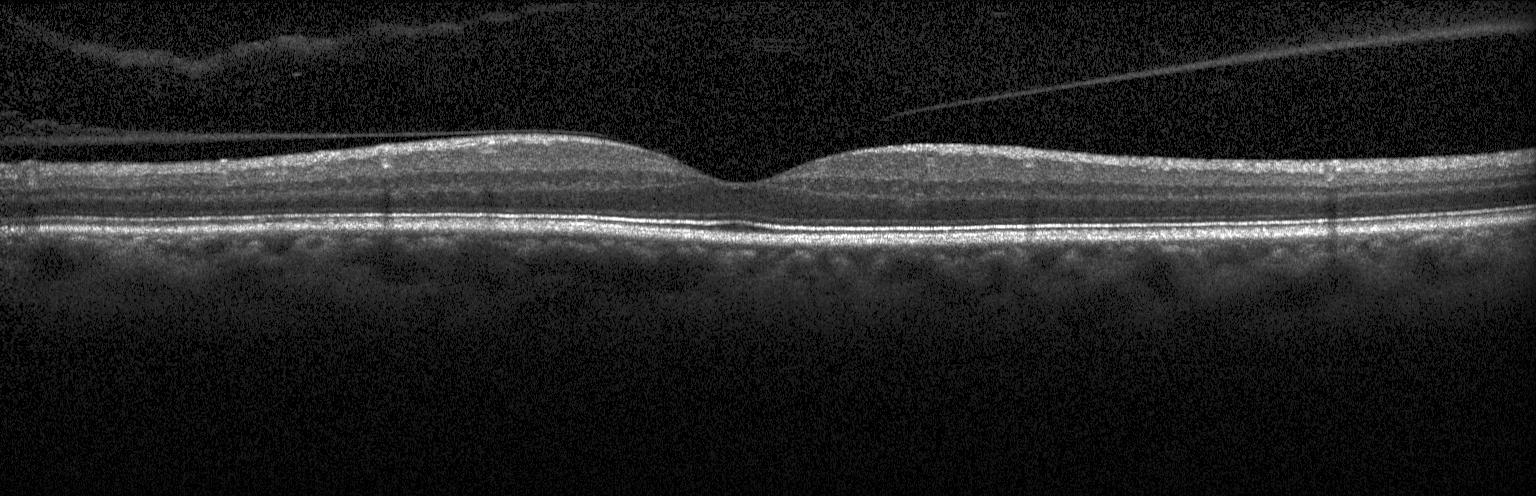

Optical coherence tomography scan · instrument: Heidelberg Spectralis · through the macula. Finding: neither choroidal neovascularization, diabetic macular edema, nor drusen.